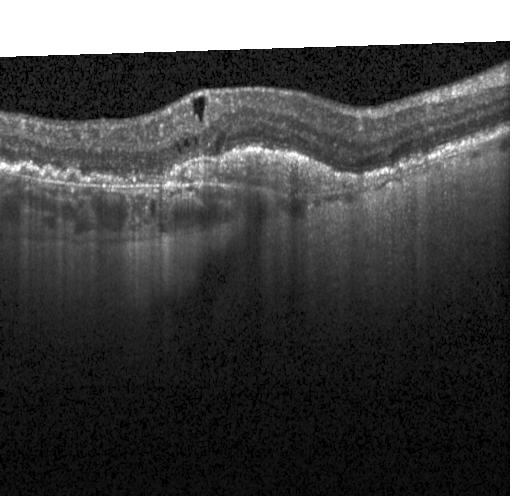 Spectral-domain OCT · OCT line scan · horizontal scan through the fovea · Heidelberg Spectralis OCT system
Diagnosis: a choroidal neovascular membrane.